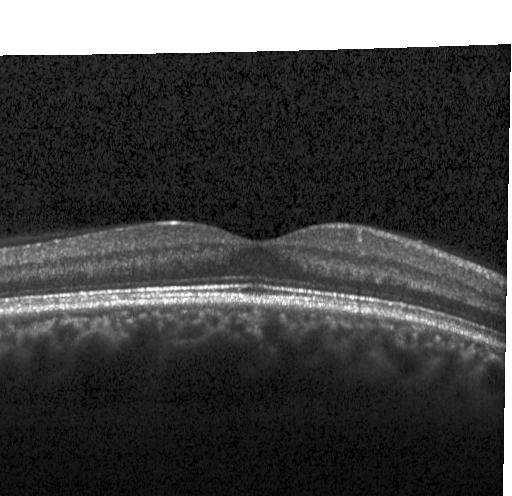 Fovea-centered. Optical coherence tomography B-scan. Assessment: no choroidal neovascularization, no diabetic macular edema, and no drusen.